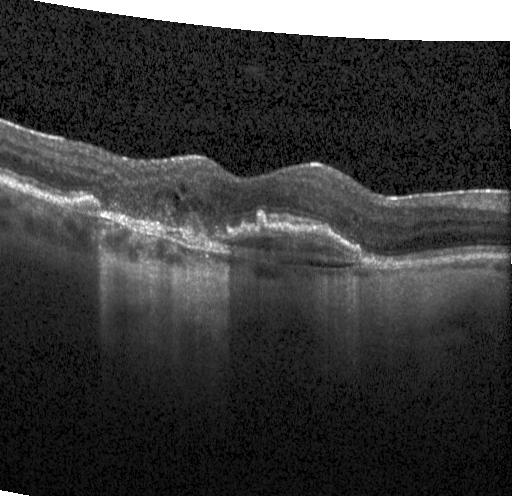

OCT B-scan showing choroidal neovascularization (CNV).